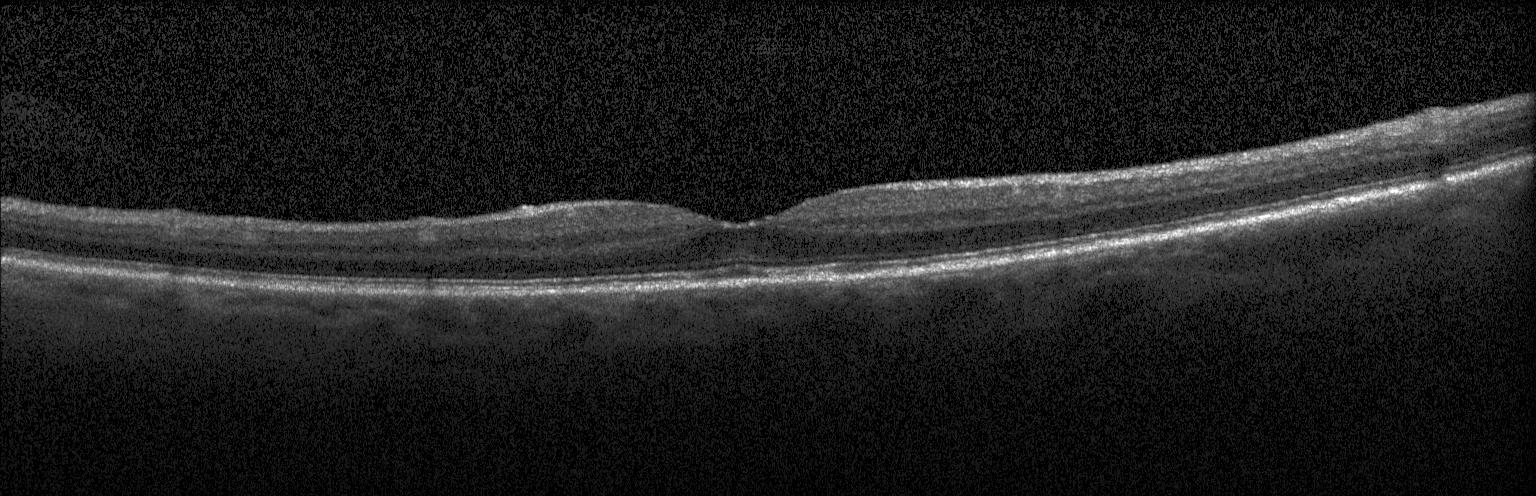

Diagnosis: neither choroidal neovascularization, diabetic macular edema, nor drusen.